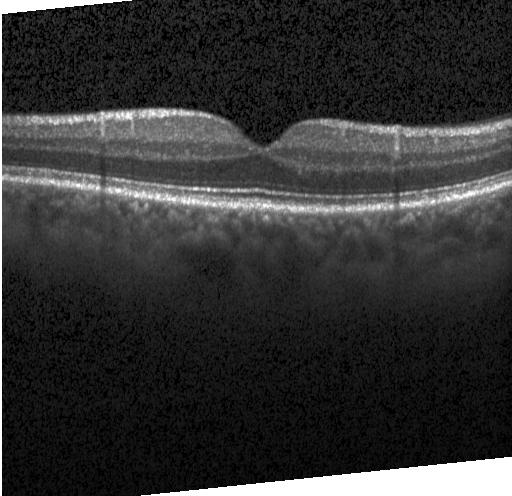

Impression: no CNV, DME, or drusen.